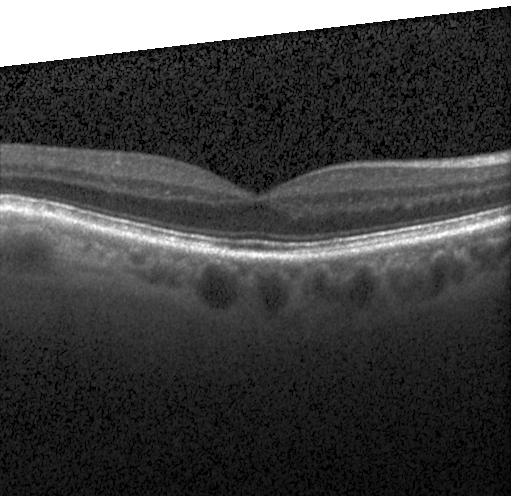 Macular scan, acquired on a Heidelberg Spectralis, spectral-domain OCT, OCT line scan.
The scan shows no choroidal neovascularization, diabetic macular edema, or drusen.